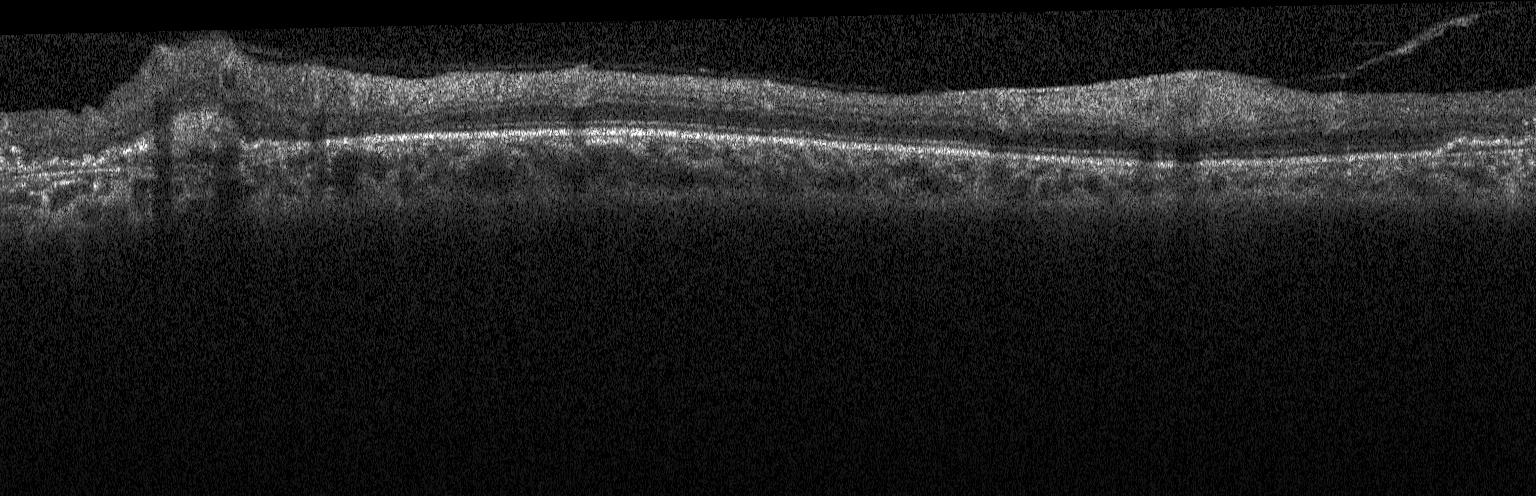
Fovea-centered, optical coherence tomography B-scan. Diagnosis: a choroidal neovascular membrane.